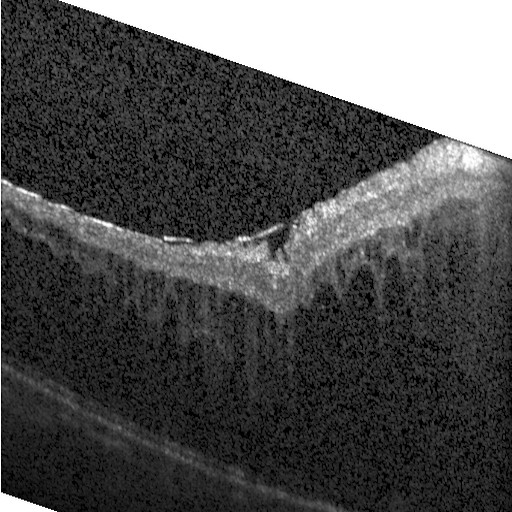
Macular scan. Heidelberg Spectralis. Spectral-domain optical coherence tomography. OCT line scan. This B-scan demonstrates diabetic macular edema (DME).